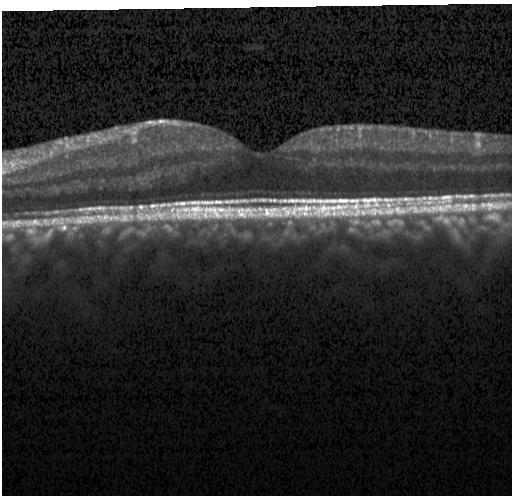

Diagnosis: no evidence of CNV, DME, or drusen.